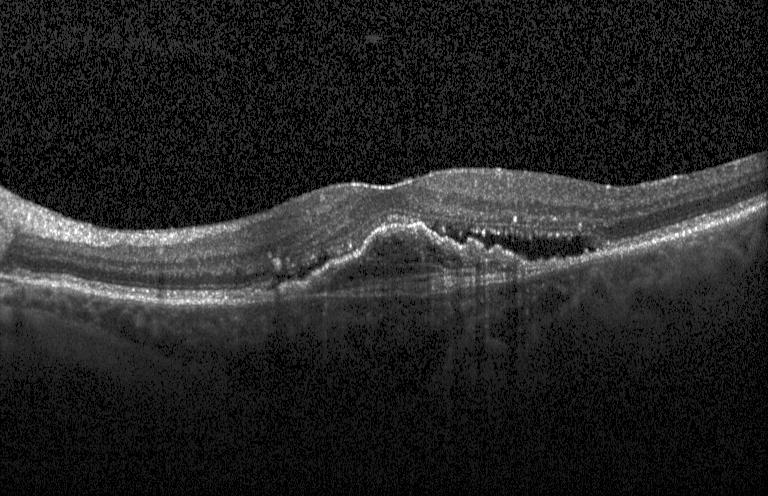 This B-scan demonstrates choroidal neovascularization (CNV).